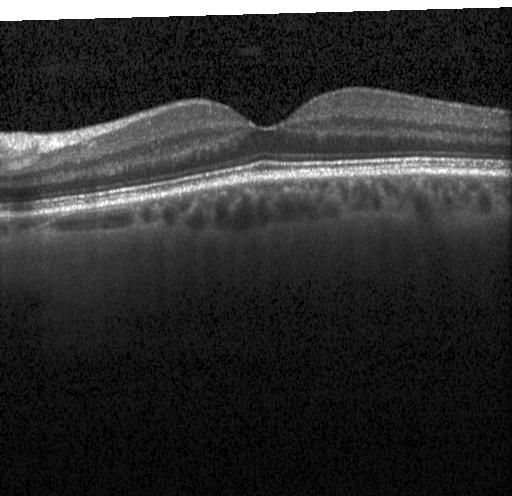

Through the macula. Optical coherence tomography B-scan. Diagnosis: no evidence of choroidal neovascularization, diabetic macular edema, or drusen.